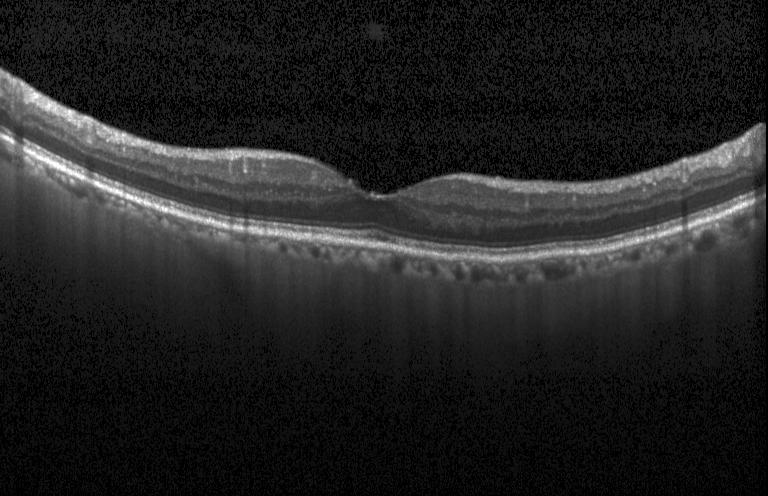
Instrument: Heidelberg Spectralis · SD-OCT · horizontal scan through the fovea · optical coherence tomography B-scan.
Diagnosis: no choroidal neovascularization, no diabetic macular edema, and no drusen.